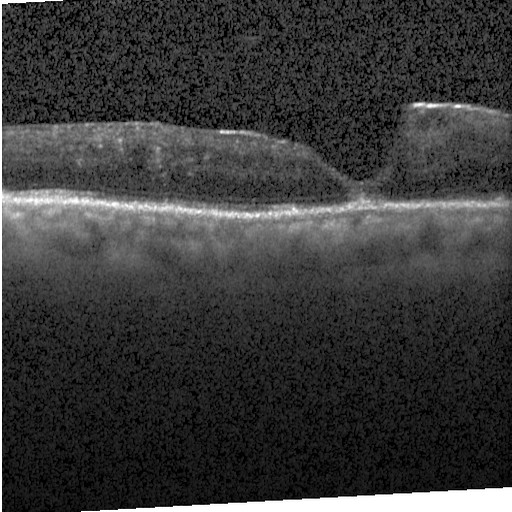

Optical coherence tomography scan; fovea-centered.
OCT finding: diabetic macular edema (DME).